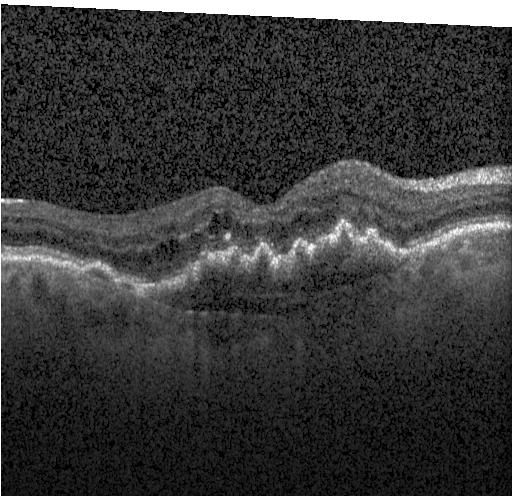 Diagnosis: a choroidal neovascular membrane.